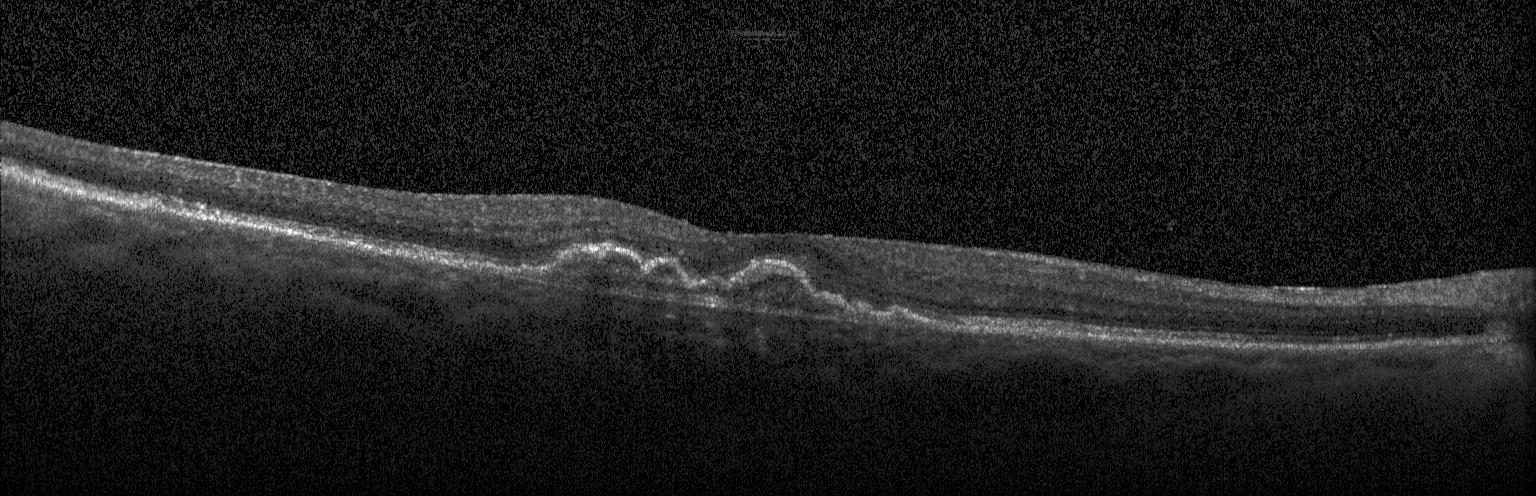

OCT finding: choroidal neovascularization (CNV).